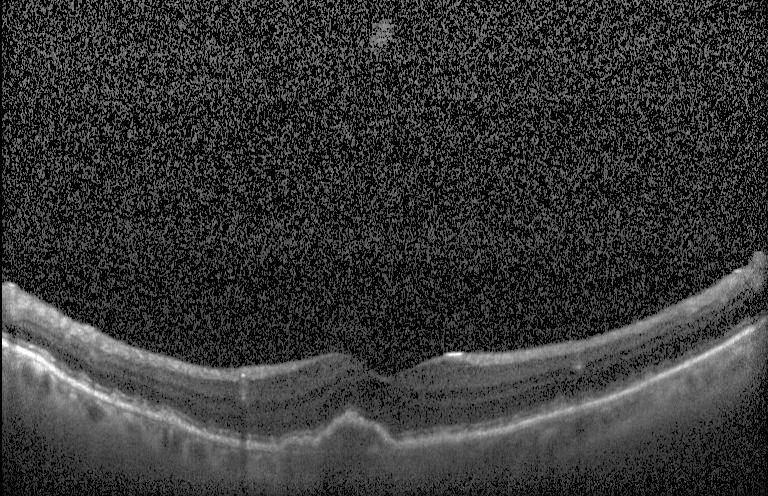
OCT line scan; Heidelberg Spectralis OCT system
Finding: choroidal neovascularization.